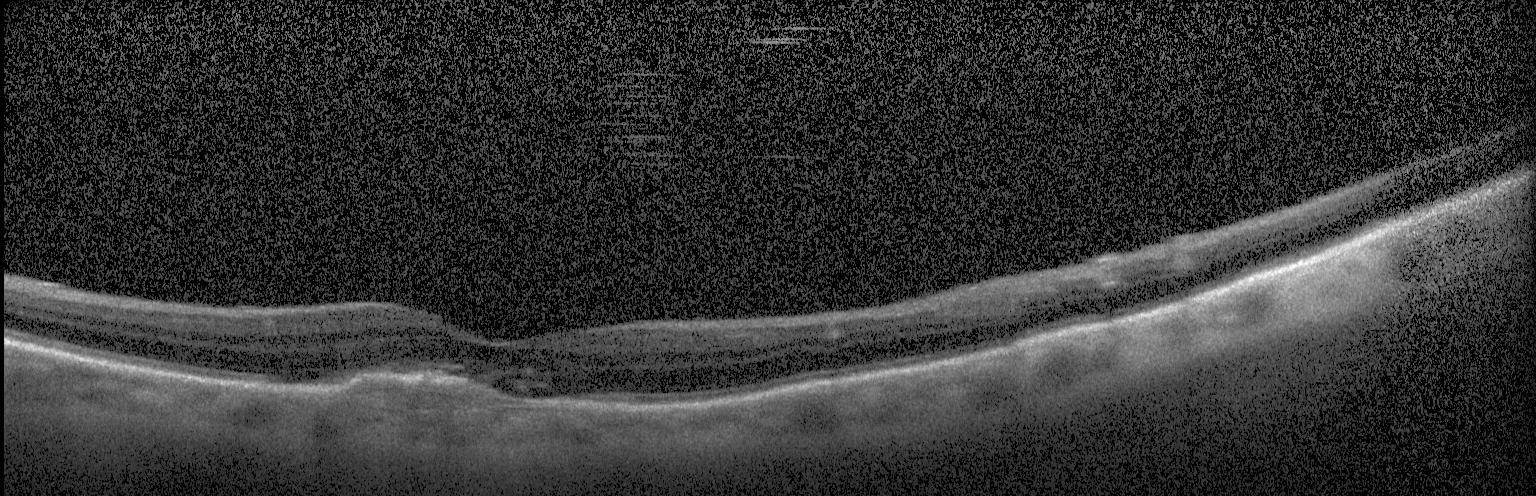
Optical coherence tomography scan, horizontal scan through the fovea — A choroidal neovascular membrane.